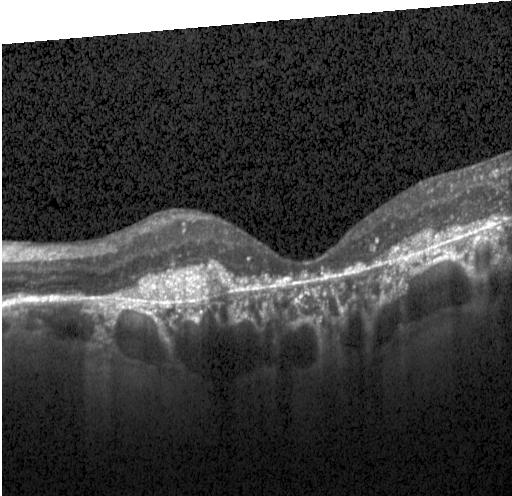

Retinal OCT cross-section, SD-OCT — Choroidal neovascularization.